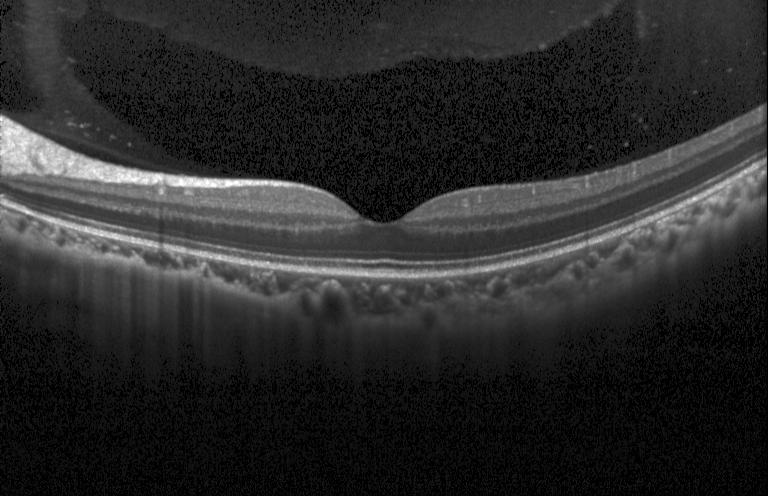 Acquired on a Heidelberg Spectralis · optical coherence tomography B-scan · SD-OCT. Impression: no choroidal neovascularization, diabetic macular edema, or drusen.